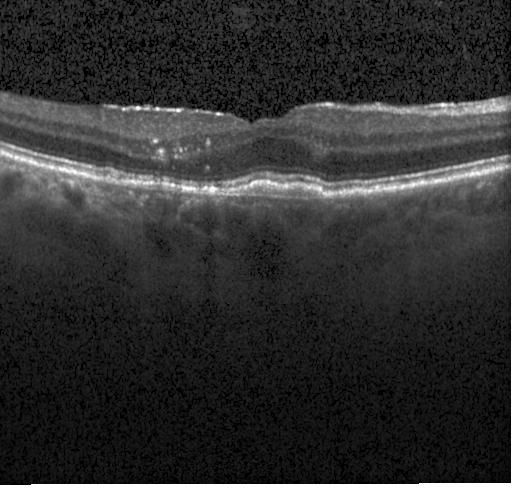

Assessment: a choroidal neovascular membrane.